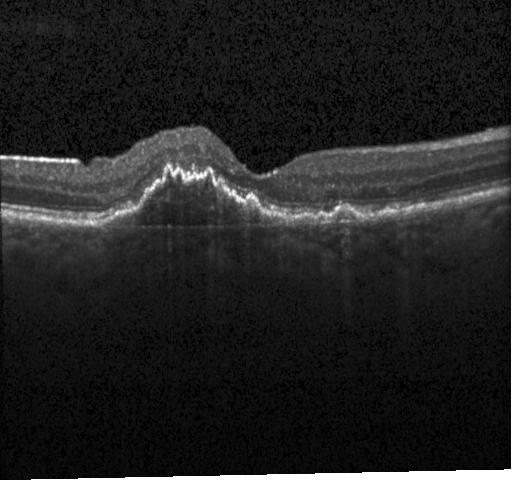
OCT B-scan; fovea-centered; spectral-domain OCT; acquired on a Heidelberg Spectralis.
The scan shows CNV.